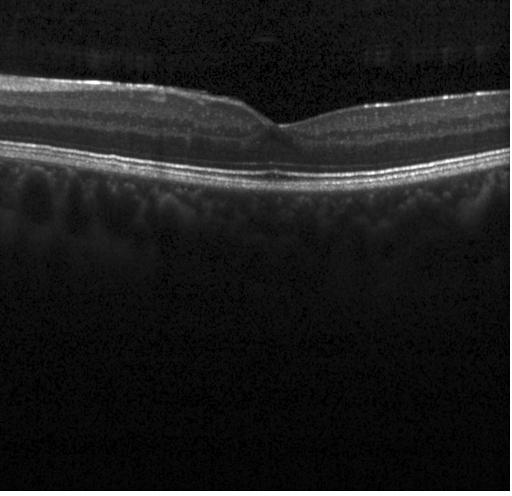 Instrument: Heidelberg Spectralis. Retinal OCT B-scan.
Finding: neither CNV, DME, nor drusen.